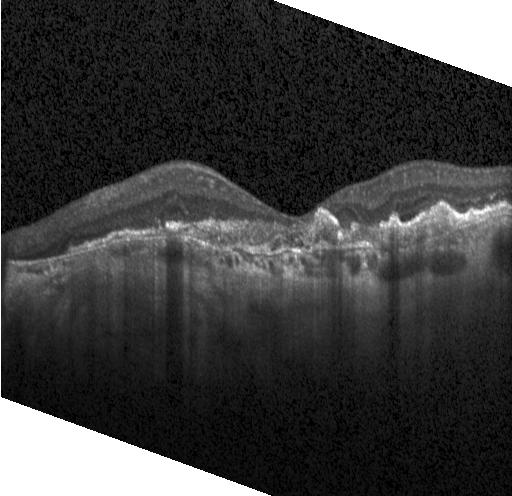 Retinal OCT B-scan · spectral-domain OCT · instrument: Heidelberg Spectralis · macular scan — Diagnosis: a choroidal neovascular membrane.